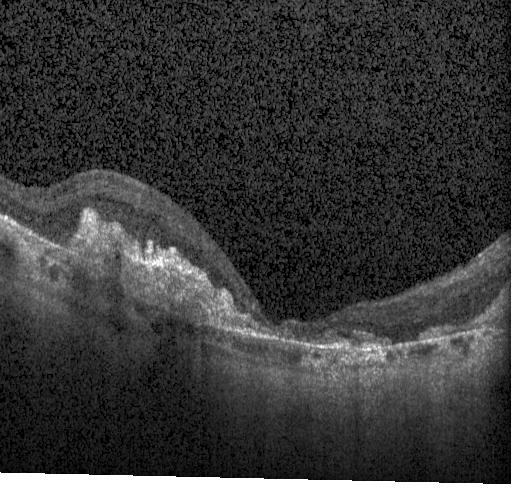 Impression: a choroidal neovascular membrane.